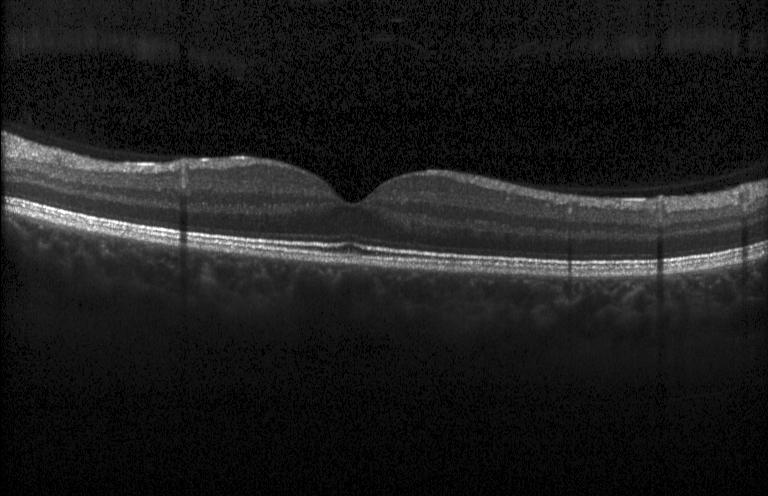 Retinal OCT B-scan — No choroidal neovascularization, no diabetic macular edema, and no drusen.